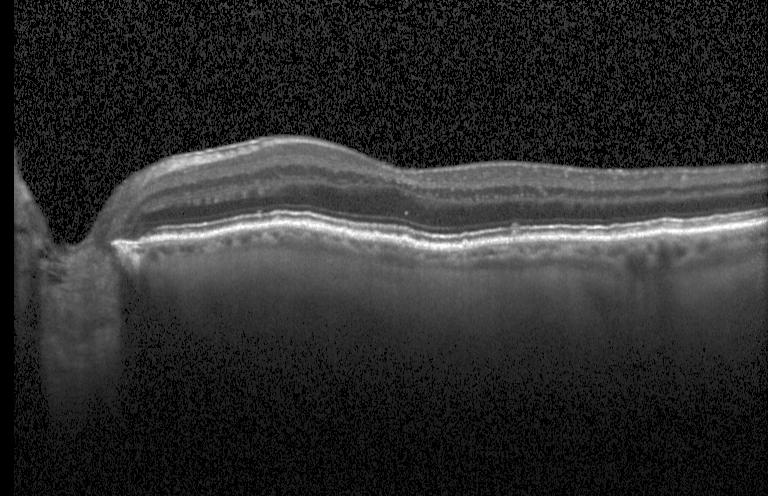
Retinal OCT cross-section · fovea-centered · Heidelberg Spectralis OCT system — This B-scan demonstrates sub-RPE drusenoid deposits.